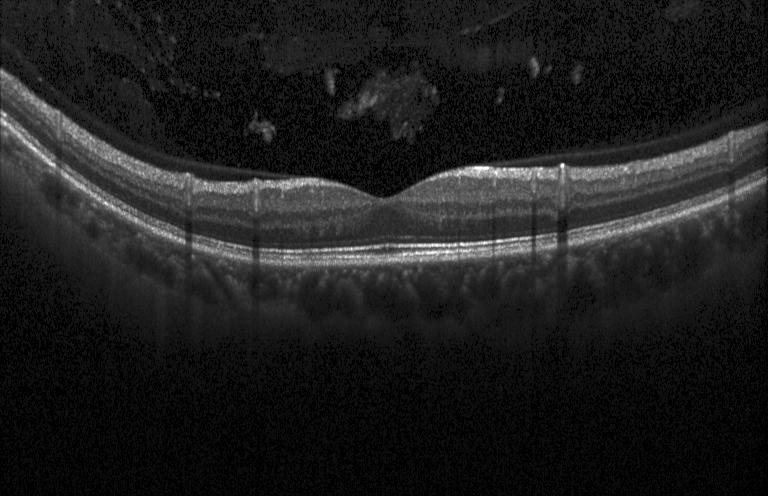
Heidelberg Spectralis OCT system · OCT line scan
Neither choroidal neovascularization, diabetic macular edema, nor drusen.